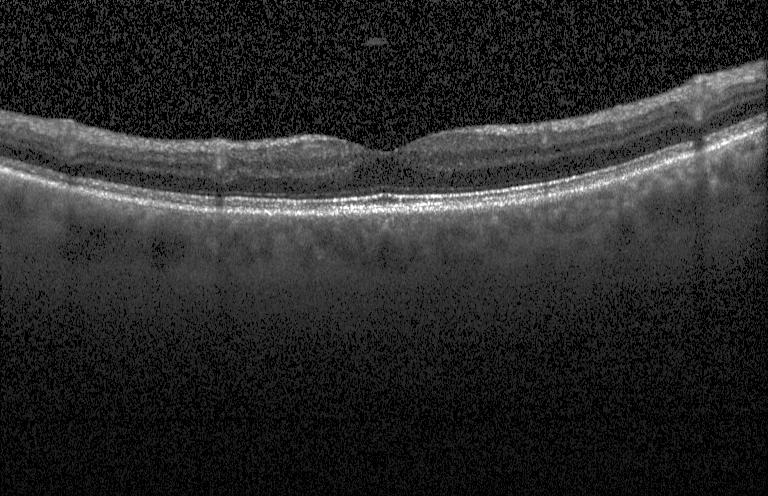

Diagnosis: no evidence of choroidal neovascularization, diabetic macular edema, or drusen.